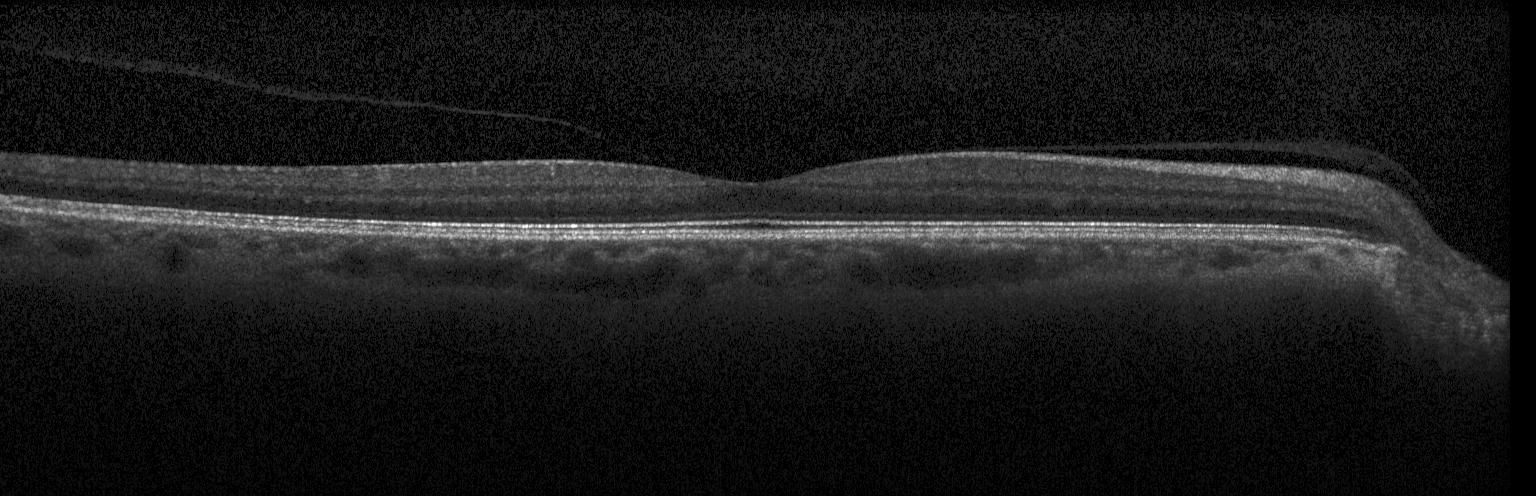

Retinal OCT B-scan — Impression: no CNV, DME, or drusen.